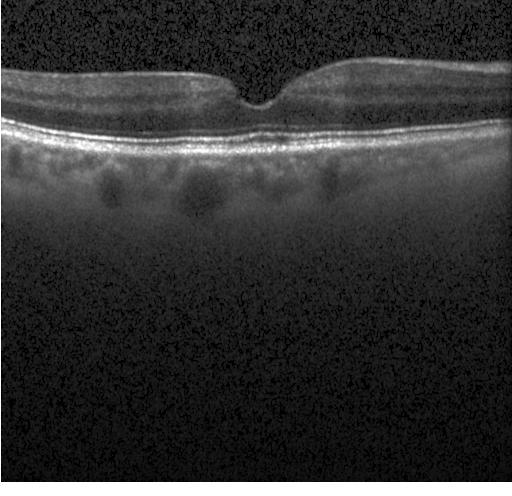
Retinal OCT B-scan
Assessment: no CNV, DME, or drusen.